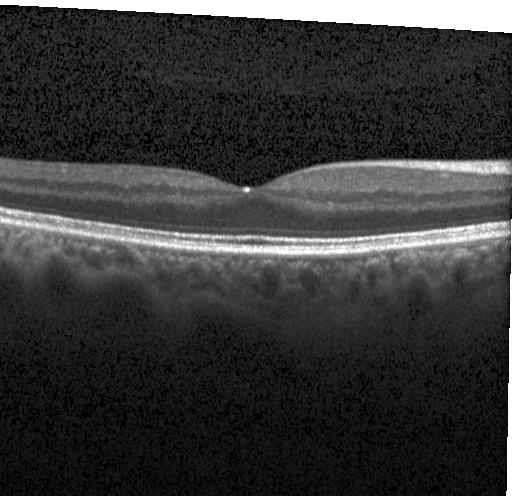
Spectral-domain OCT · retinal OCT B-scan · centered on the fovea. Dx: no choroidal neovascularization, no diabetic macular edema, and no drusen.